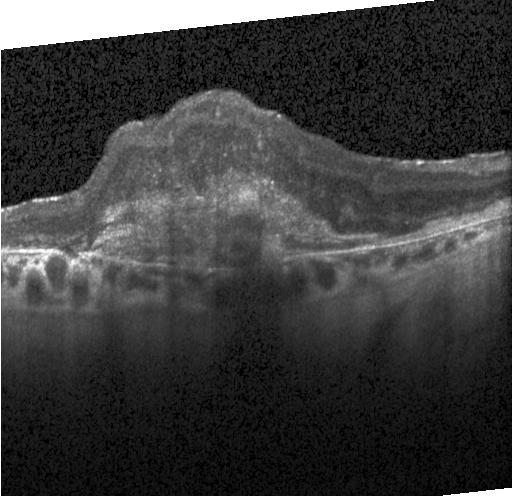

Retinal OCT B-scan
OCT finding: a choroidal neovascular membrane.